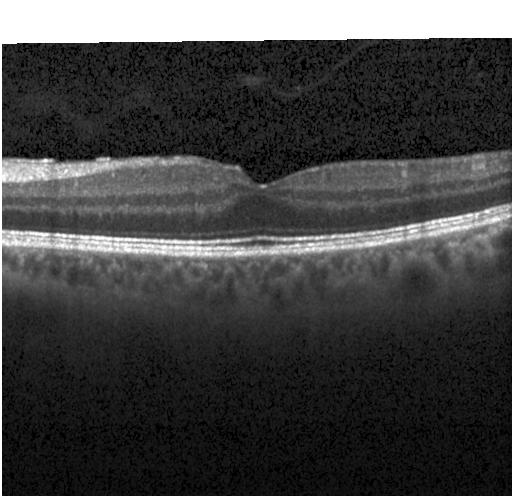 Spectral-domain OCT B-scan: no CNV, no DME, and no drusen.